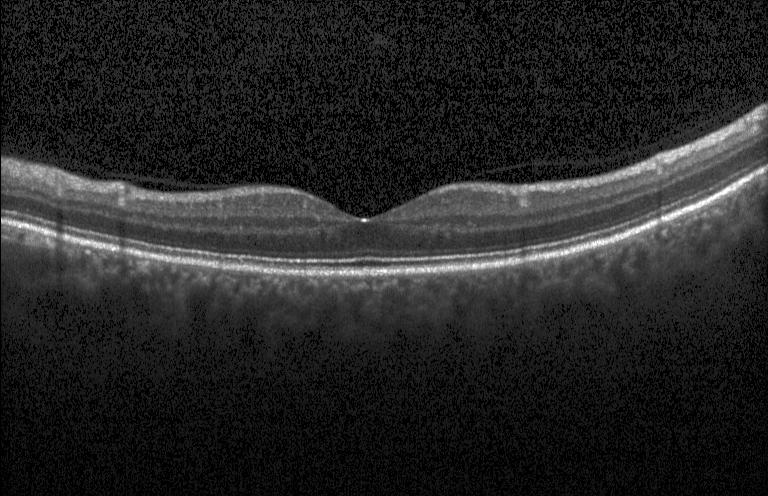
No choroidal neovascularization, diabetic macular edema, or drusen.